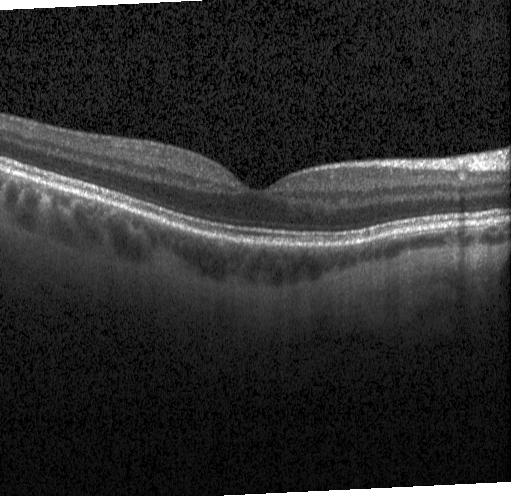
Retinal OCT cross-section showing no CNV, no DME, and no drusen.